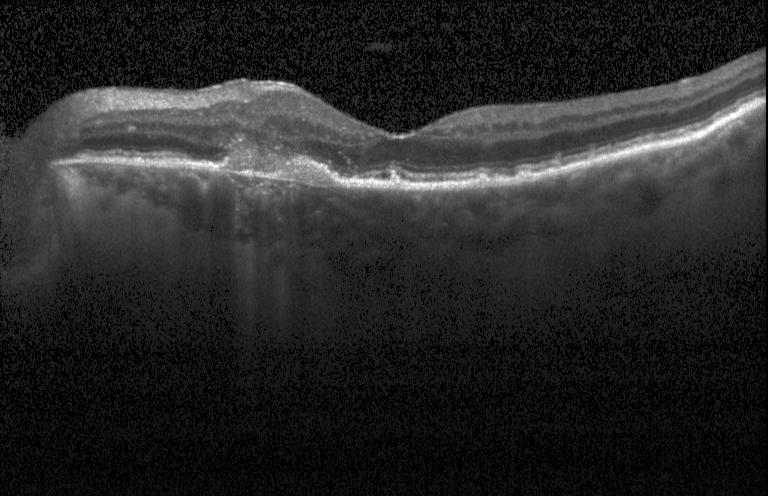 Acquired on a Heidelberg Spectralis; optical coherence tomography B-scan
Impression: a choroidal neovascular membrane.